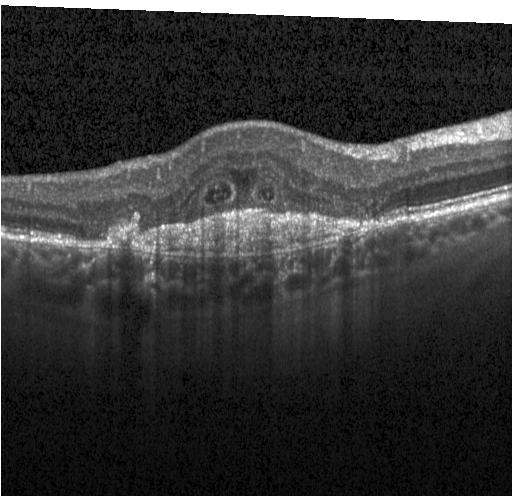
Retinal OCT cross-section. Diagnosis: a choroidal neovascular membrane.